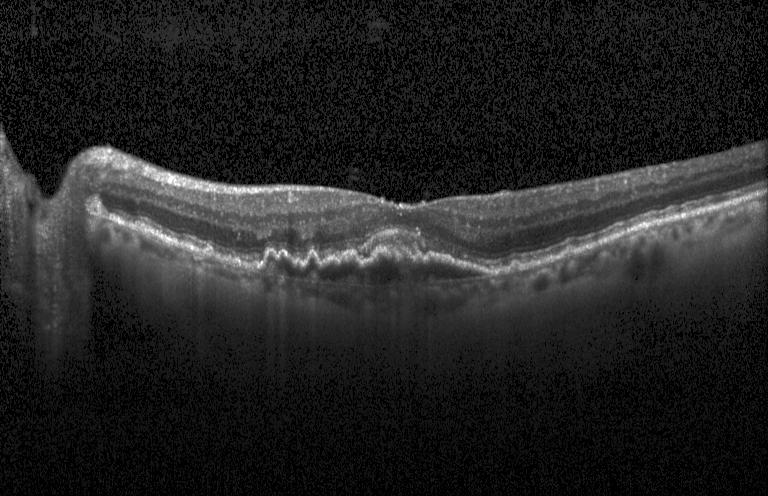
Dx: CNV.